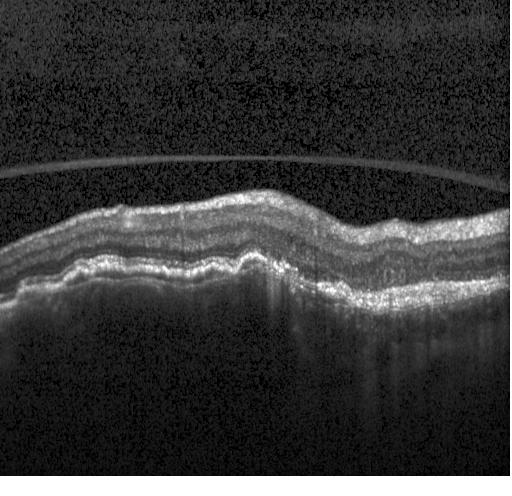 Spectral-domain optical coherence tomography; OCT B-scan; fovea-centered — Impression: choroidal neovascularization.